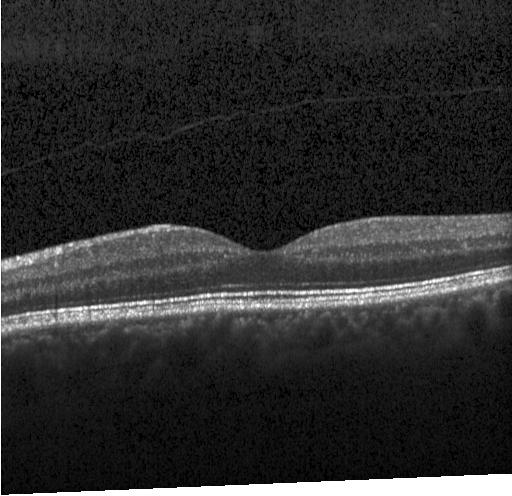 OCT line scan — OCT finding: no CNV, DME, or drusen.